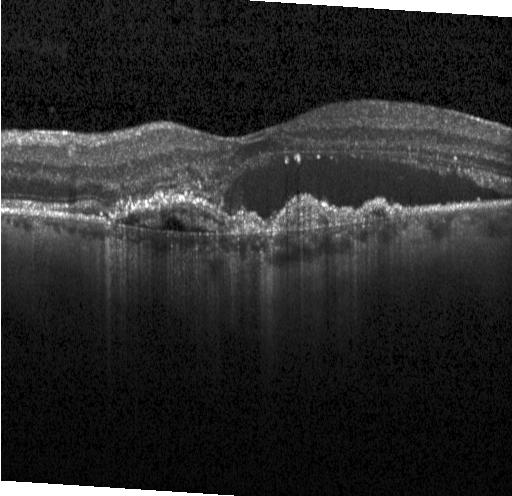
Retinal OCT B-scan · spectral-domain OCT · macular scan · instrument: Heidelberg Spectralis.
Impression: a choroidal neovascular membrane.